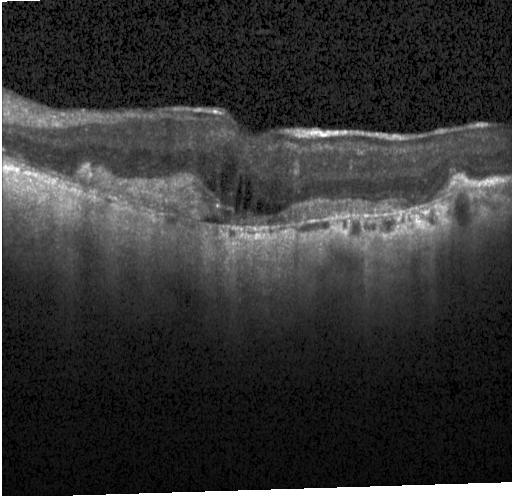 Fovea-centered, spectral-domain optical coherence tomography, OCT B-scan, instrument: Heidelberg Spectralis
OCT finding: a choroidal neovascular membrane.